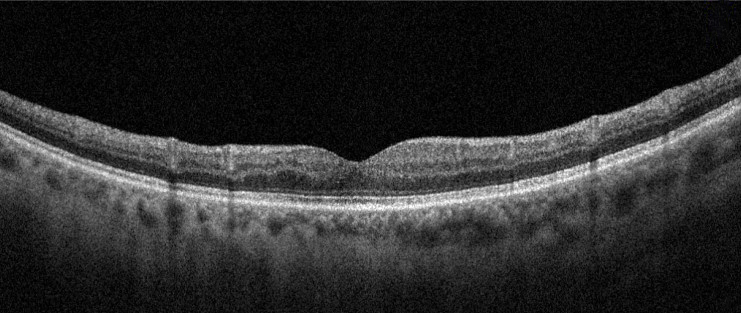

OCT finding: retinal vein occlusion (RVO).